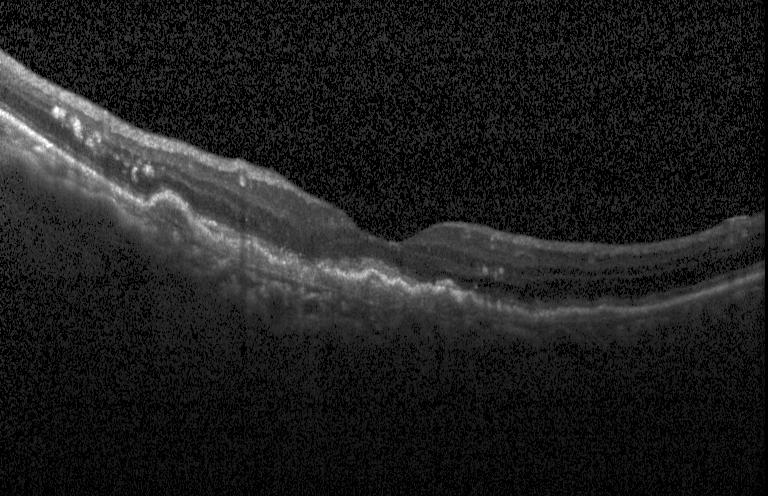

OCT line scan. Heidelberg Spectralis. Spectral-domain OCT
Assessment: a choroidal neovascular membrane.